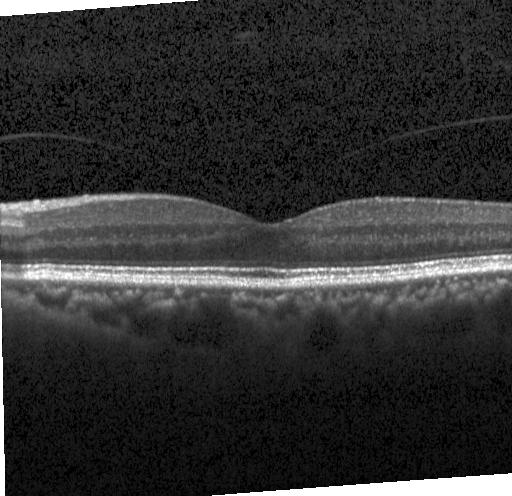 OCT line scan; spectral-domain optical coherence tomography. Diagnosis: no choroidal neovascularization, no diabetic macular edema, and no drusen.